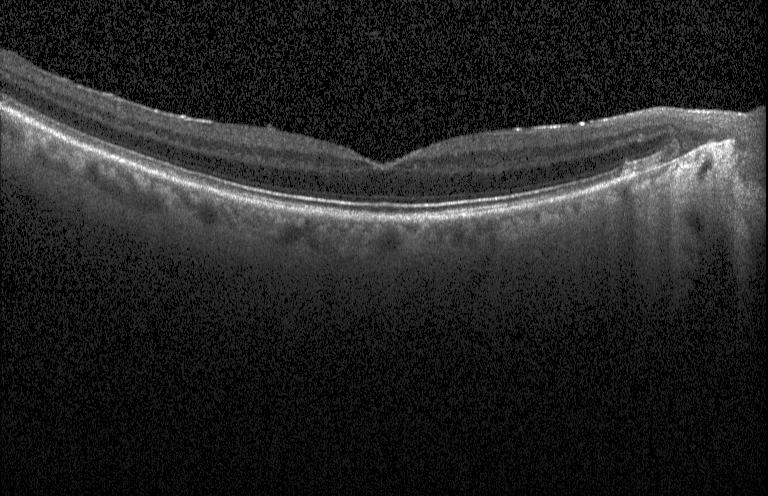

Through the macula · acquired on a Heidelberg Spectralis · retinal OCT B-scan.
Impression: no choroidal neovascularization, diabetic macular edema, or drusen.